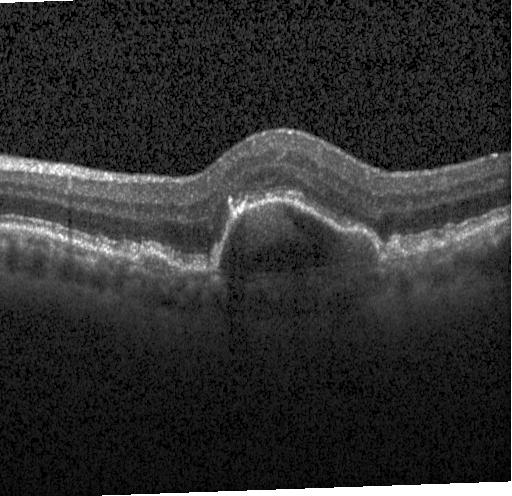 Optical coherence tomography B-scan, Heidelberg Spectralis. OCT finding: sub-RPE drusenoid deposits.